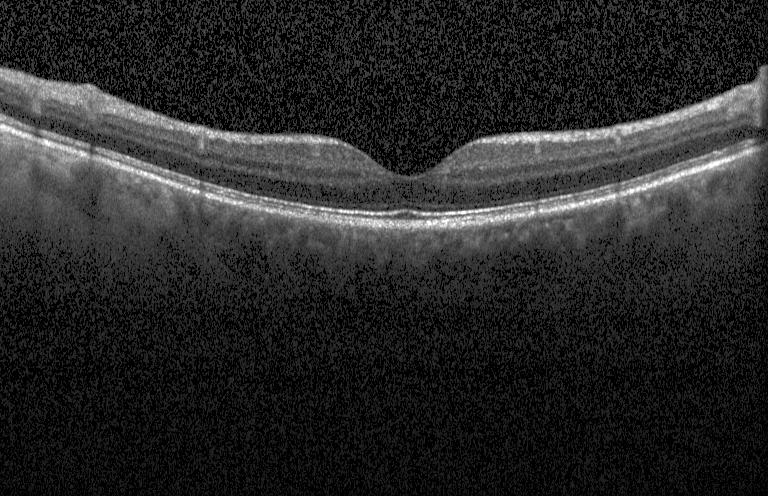

Retinal OCT cross-section — Assessment: neither choroidal neovascularization, diabetic macular edema, nor drusen.